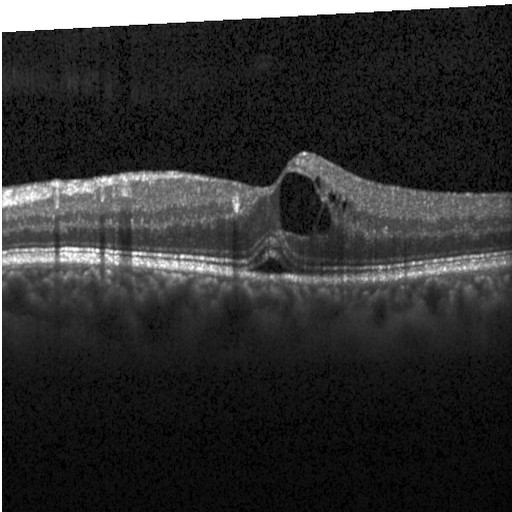 Macular scan; OCT line scan
Finding: diabetic macular edema (DME).